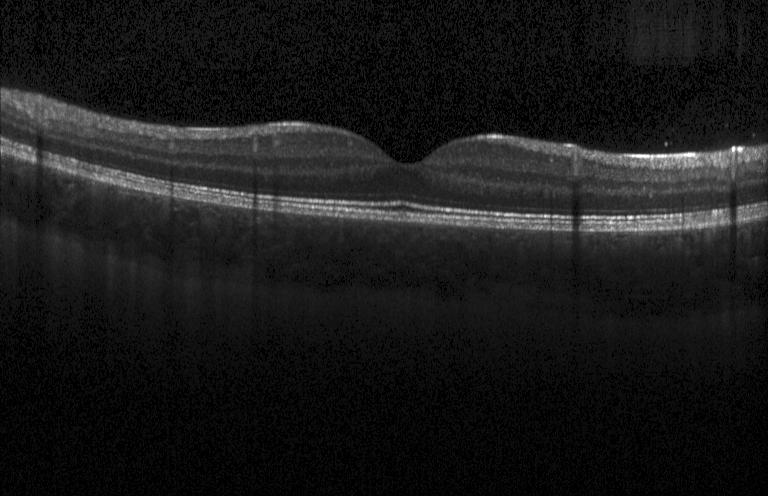

Spectral-domain OCT B-scan: no choroidal neovascularization, no diabetic macular edema, and no drusen.